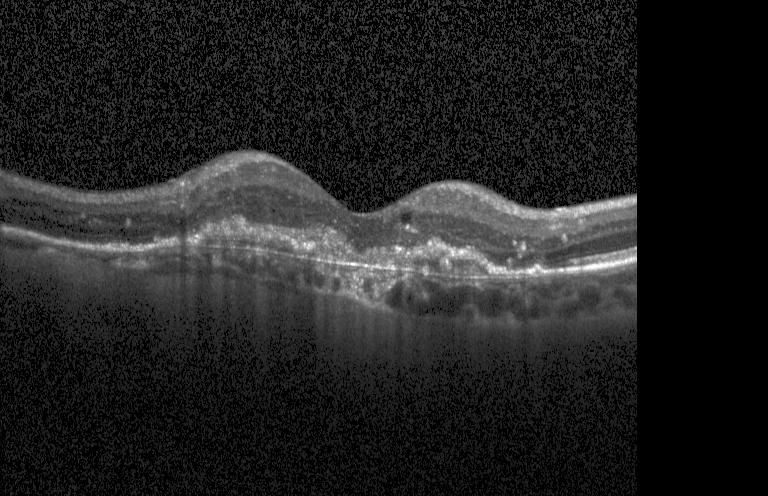
Macular OCT: choroidal neovascularization.